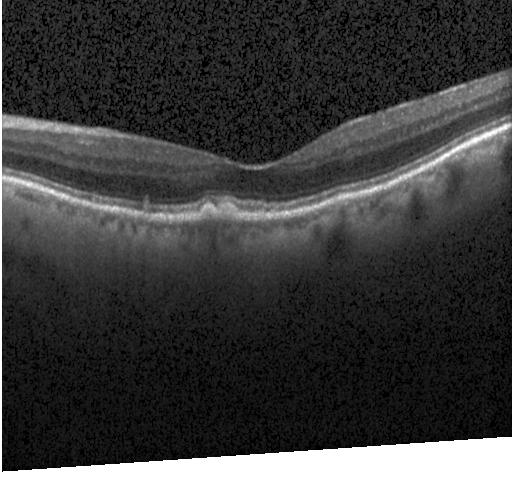

Retinal OCT B-scan. Centered on the fovea — Assessment: sub-RPE drusenoid deposits.